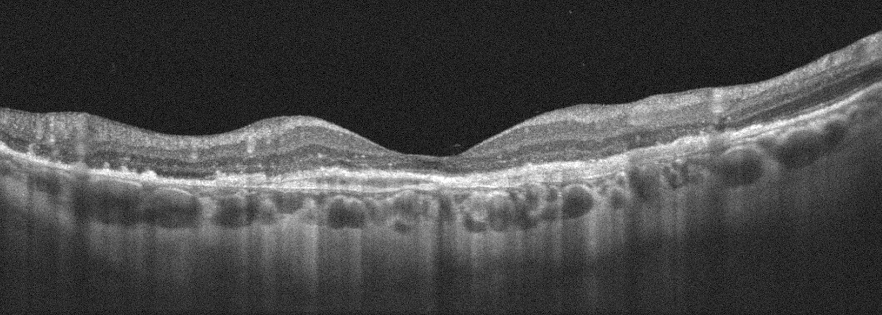

OS, retinal OCT cross-section
Diagnosis: AMD.